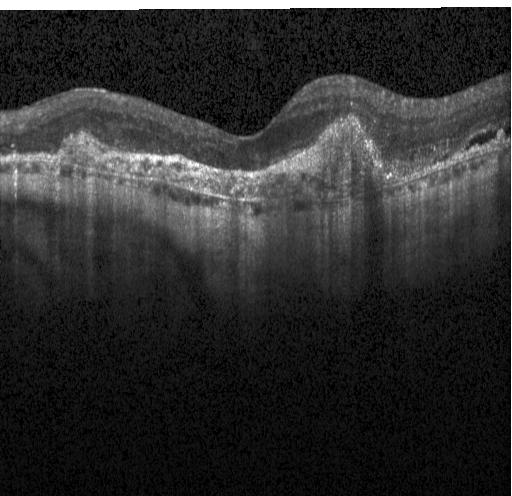

Optical coherence tomography scan. Fovea-centered — Choroidal neovascularization.